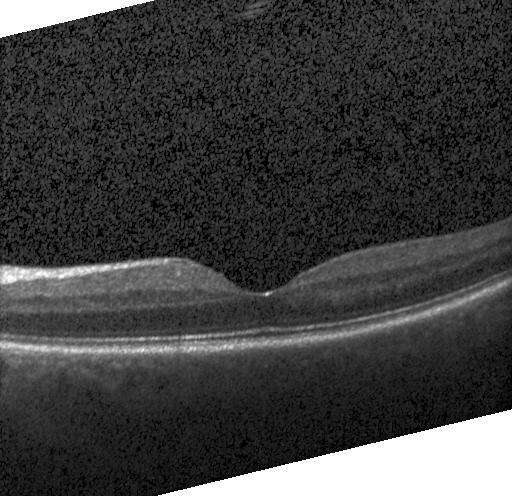
The scan shows no evidence of choroidal neovascularization, diabetic macular edema, or drusen.